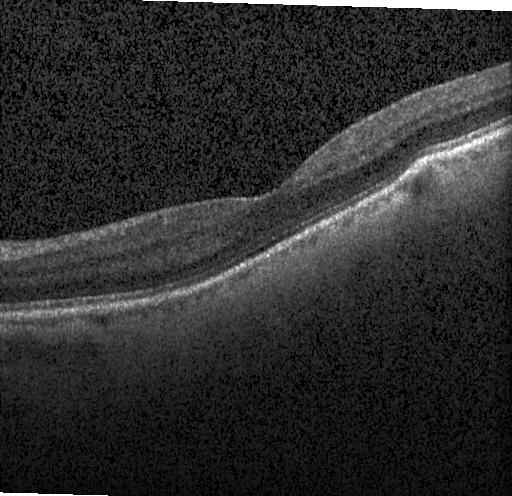

Heidelberg Spectralis · spectral-domain optical coherence tomography · retinal OCT cross-section — No evidence of CNV, DME, or drusen.